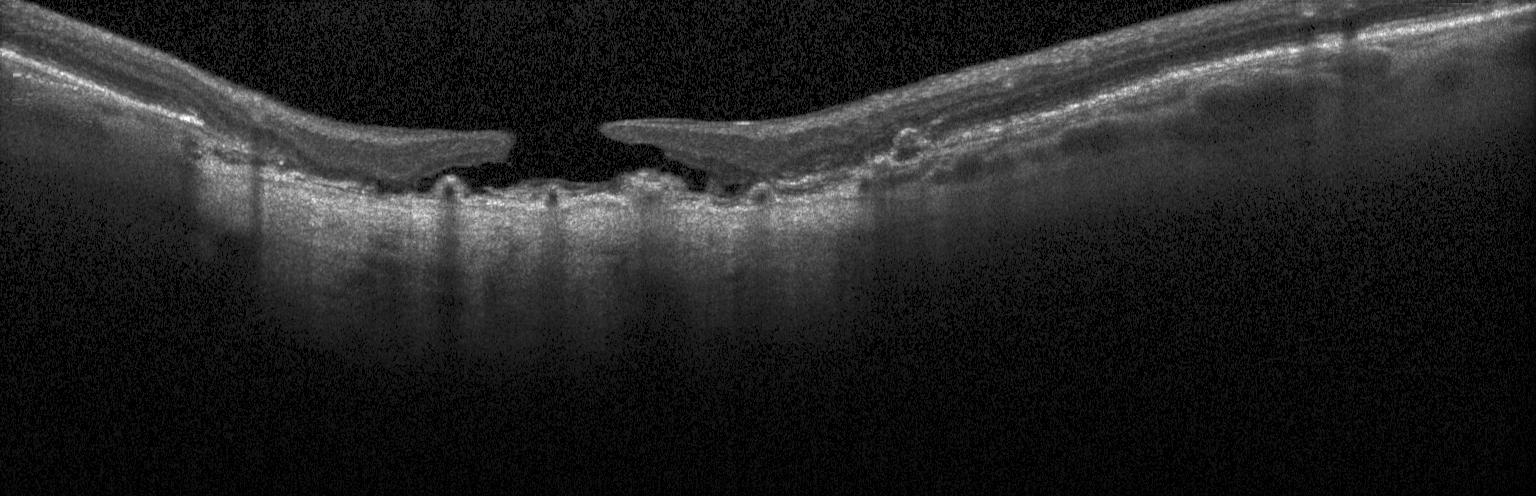
A choroidal neovascular membrane.